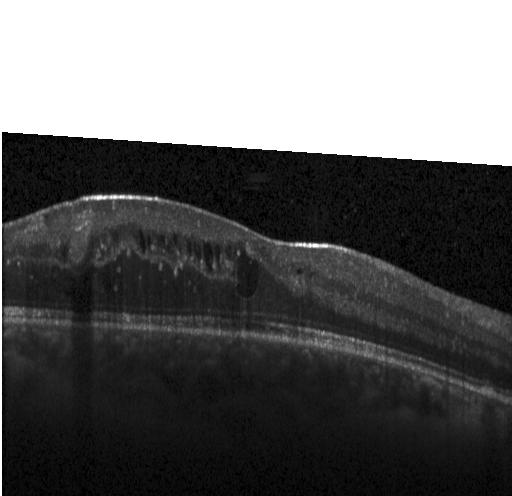 Spectral-domain optical coherence tomography · Heidelberg Spectralis OCT system · optical coherence tomography scan.
Diagnosis: diabetic macular edema (DME).